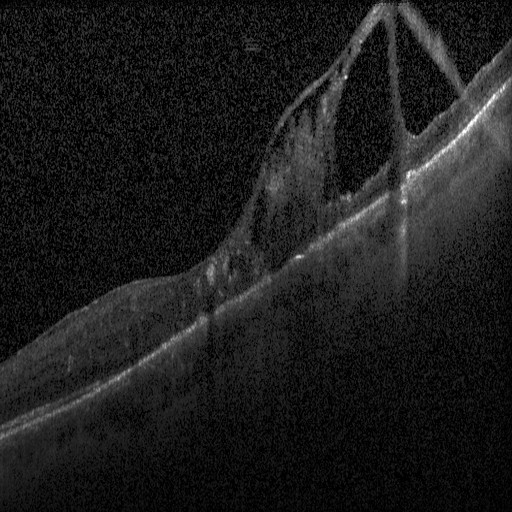

Spectral-domain OCT B-scan: DME.